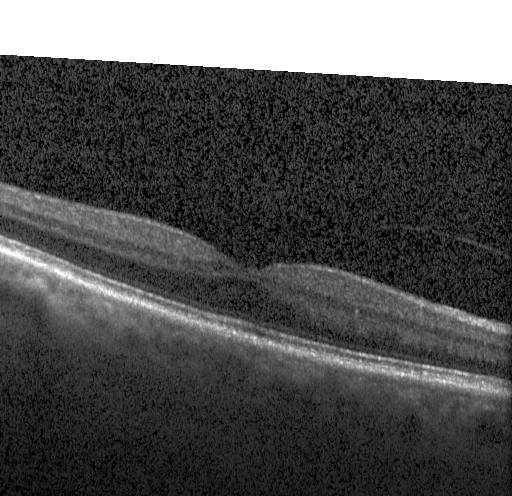

Spectral-domain OCT · fovea-centered · OCT line scan · instrument: Heidelberg Spectralis.
Impression: neither choroidal neovascularization, diabetic macular edema, nor drusen.